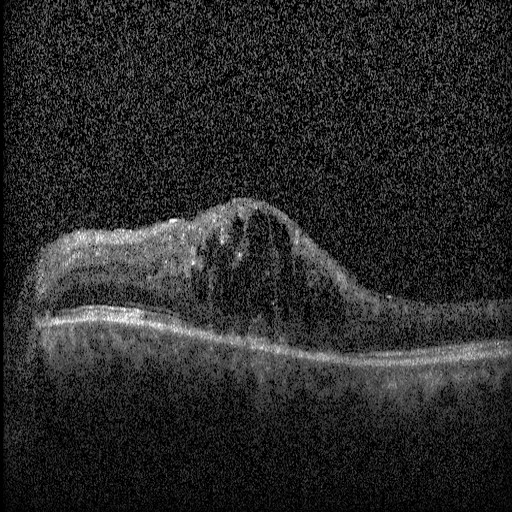
OCT finding: diabetic macular edema (DME).